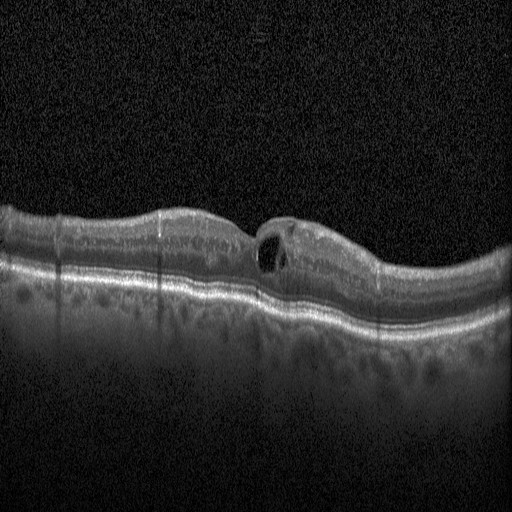 OCT line scan, spectral-domain optical coherence tomography, instrument: Heidelberg Spectralis. Macular OCT: diabetic macular edema (DME).